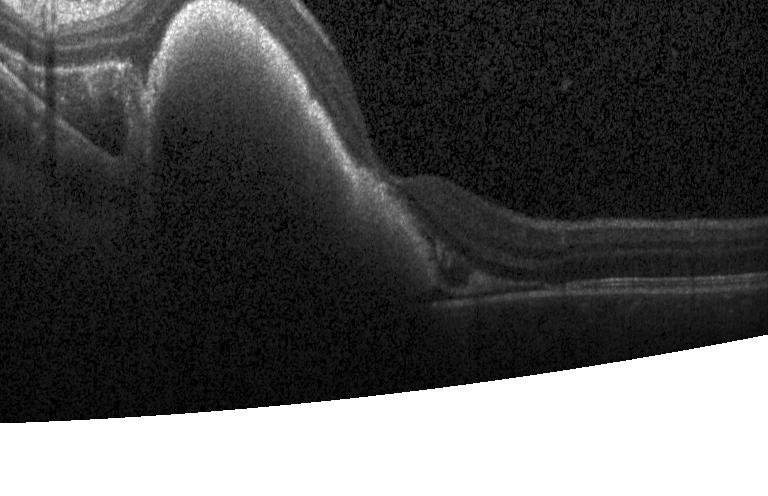

Retinal OCT B-scan; centered on the fovea; spectral-domain optical coherence tomography; instrument: Heidelberg Spectralis
Assessment: choroidal neovascularization (CNV).